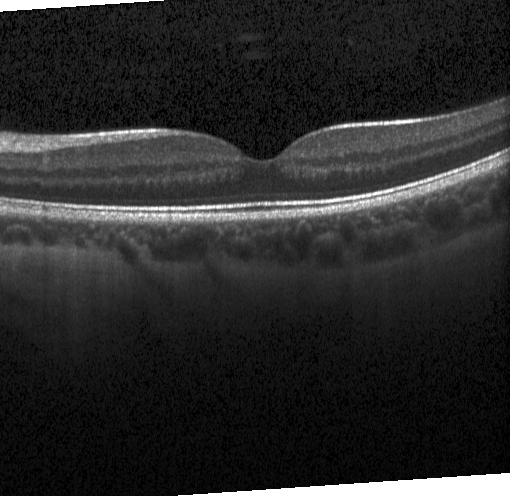 Heidelberg Spectralis OCT system. Retinal OCT B-scan. Neither choroidal neovascularization, diabetic macular edema, nor drusen.